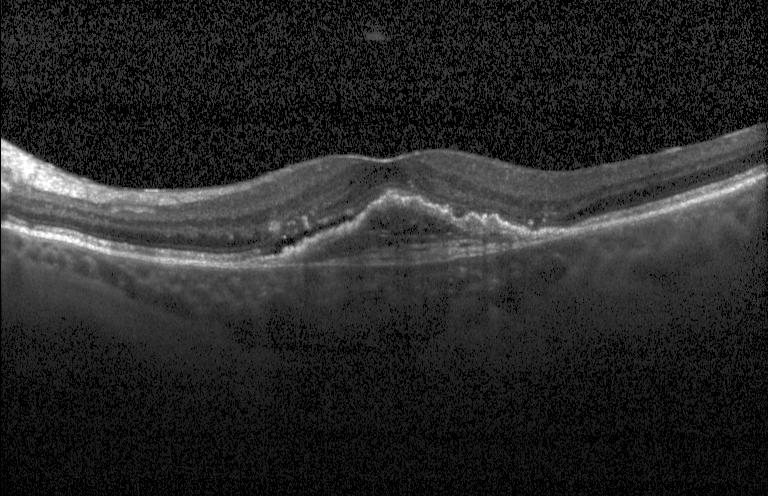 This B-scan demonstrates choroidal neovascularization.